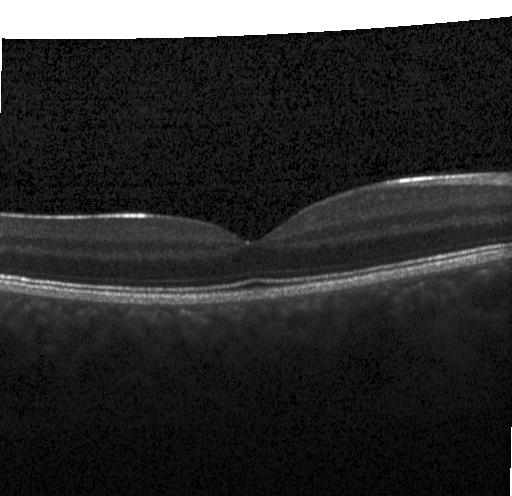

Horizontal scan through the fovea · SD-OCT · optical coherence tomography scan · Heidelberg Spectralis OCT system
Impression: neither choroidal neovascularization, diabetic macular edema, nor drusen.